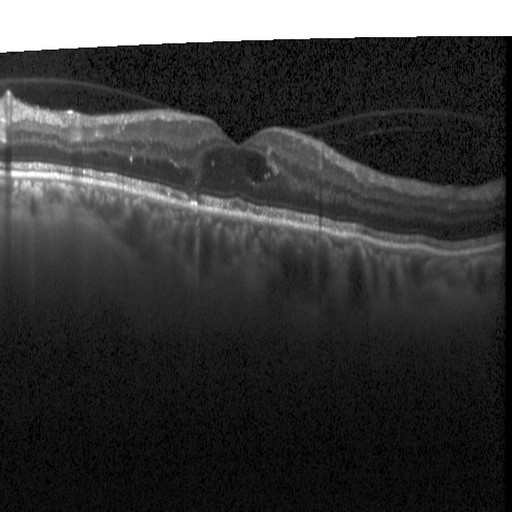 Impression: diabetic macular edema.